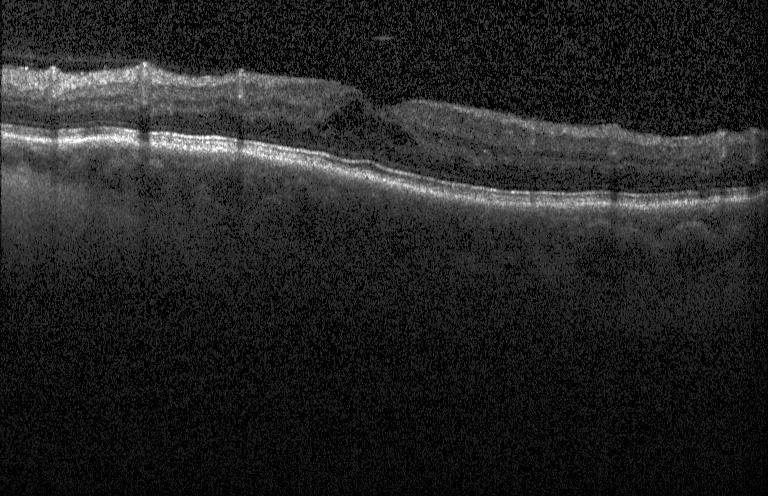 Retinal OCT cross-section, macular scan — Impression: DME.